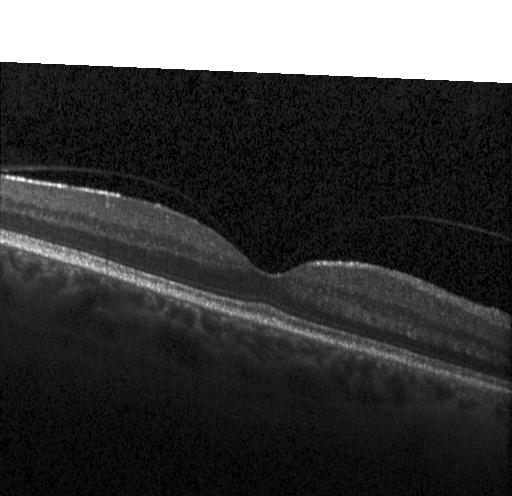
Instrument: Heidelberg Spectralis, macular scan, OCT B-scan, SD-OCT
Finding: no evidence of choroidal neovascularization, diabetic macular edema, or drusen.